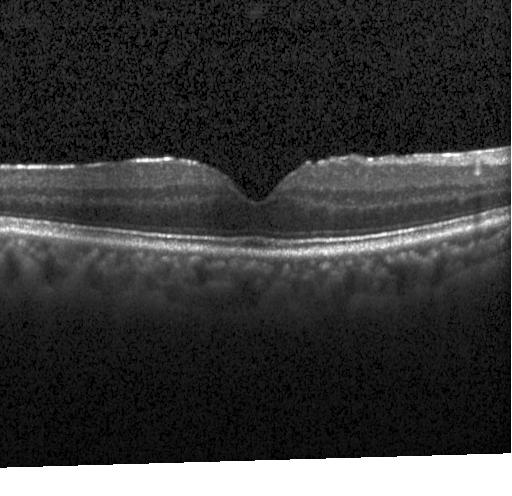
Spectral-domain OCT. Optical coherence tomography scan — Diagnosis: no choroidal neovascularization, diabetic macular edema, or drusen.